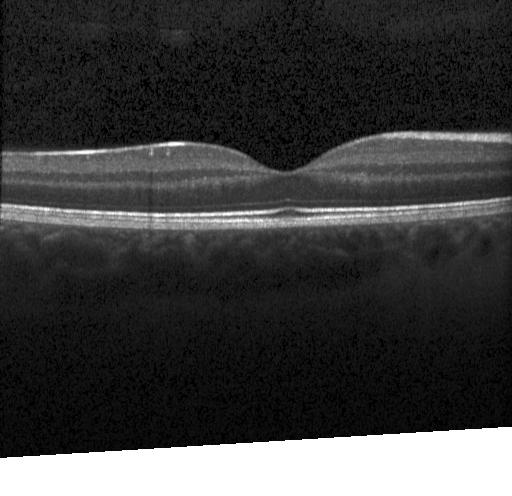

Heidelberg Spectralis OCT system · centered on the fovea · spectral-domain optical coherence tomography · OCT line scan
Macular OCT: neither CNV, DME, nor drusen.